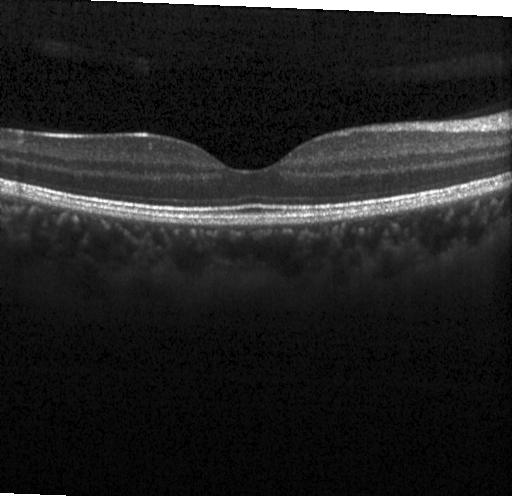

Optical coherence tomography scan; horizontal scan through the fovea. Dx: neither choroidal neovascularization, diabetic macular edema, nor drusen.